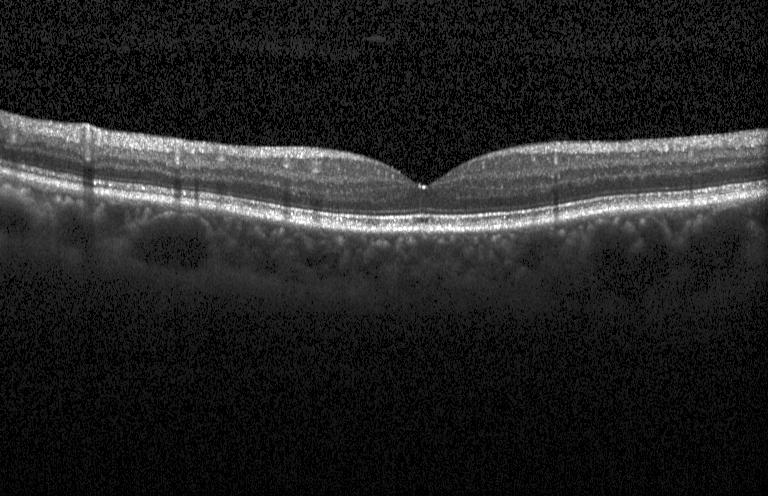 Impression: no evidence of choroidal neovascularization, diabetic macular edema, or drusen.